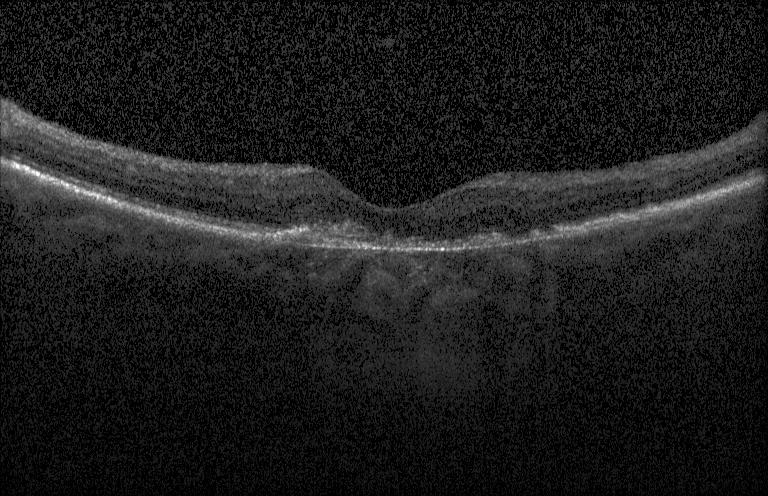

OCT B-scan · through the macula.
Impression: choroidal neovascularization (CNV).